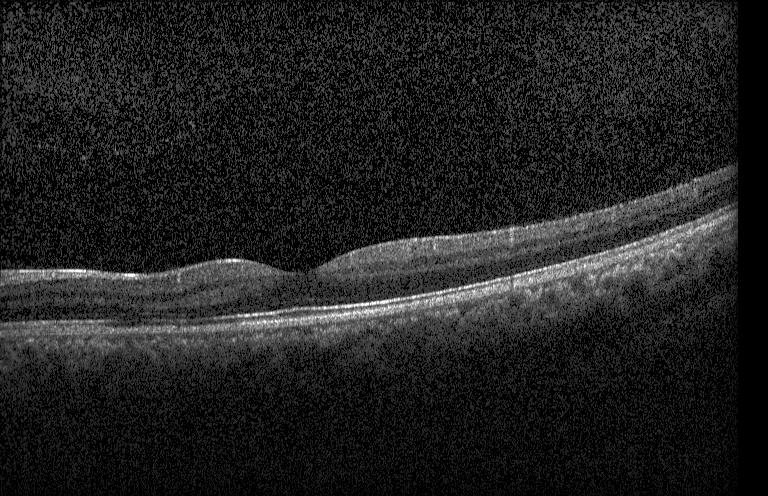
Retinal OCT B-scan.
Impression: no CNV, DME, or drusen.